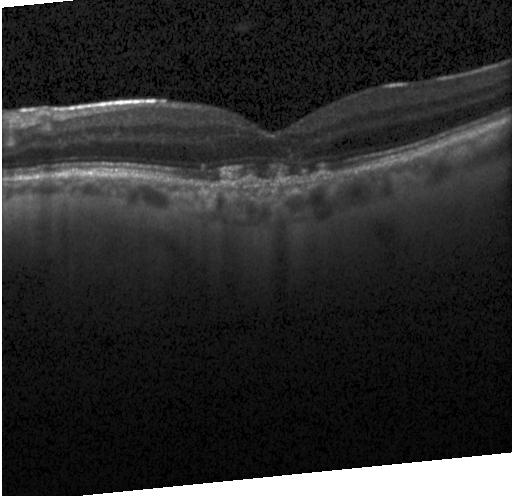

OCT B-scan, Heidelberg Spectralis OCT system, SD-OCT.
This B-scan demonstrates a choroidal neovascular membrane.